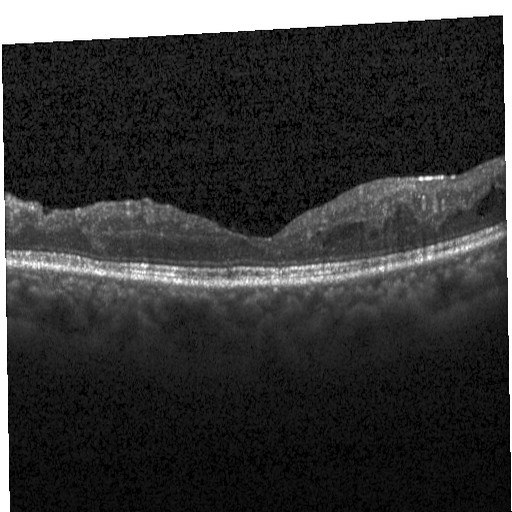

OCT line scan. Spectral-domain OCT. Macular scan. Heidelberg Spectralis OCT system. Diagnosis: DME.